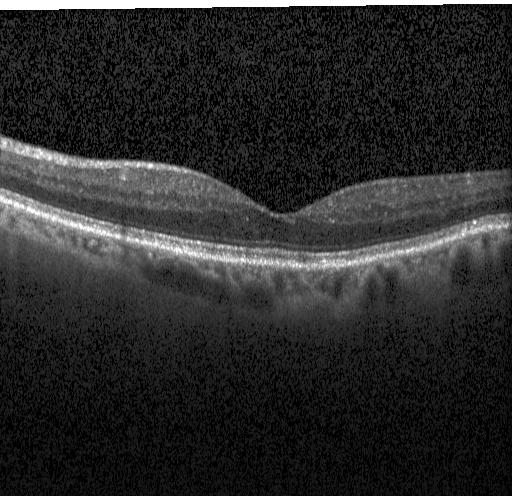 Finding: no choroidal neovascularization, diabetic macular edema, or drusen.